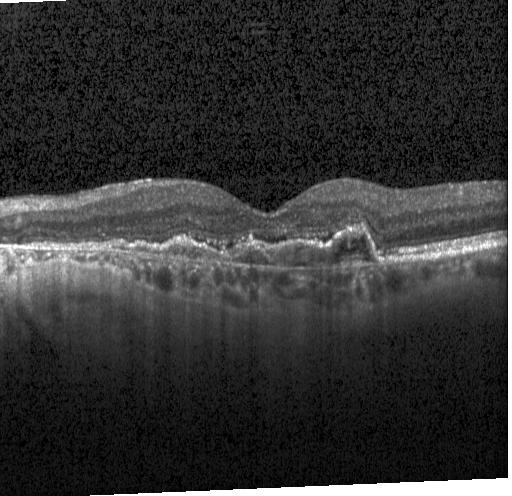 Spectral-domain OCT. Instrument: Heidelberg Spectralis. Centered on the fovea. Retinal OCT cross-section. Impression: a choroidal neovascular membrane.